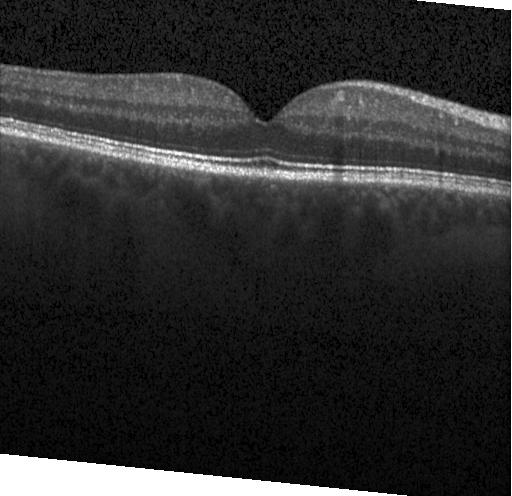

OCT B-scan showing no choroidal neovascularization, diabetic macular edema, or drusen.